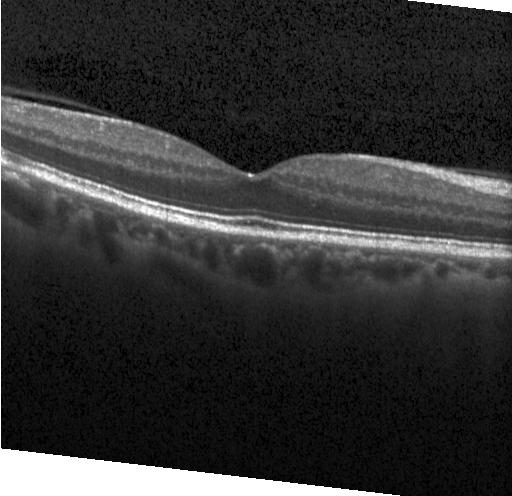

OCT line scan; spectral-domain OCT; Heidelberg Spectralis. Impression: no evidence of CNV, DME, or drusen.